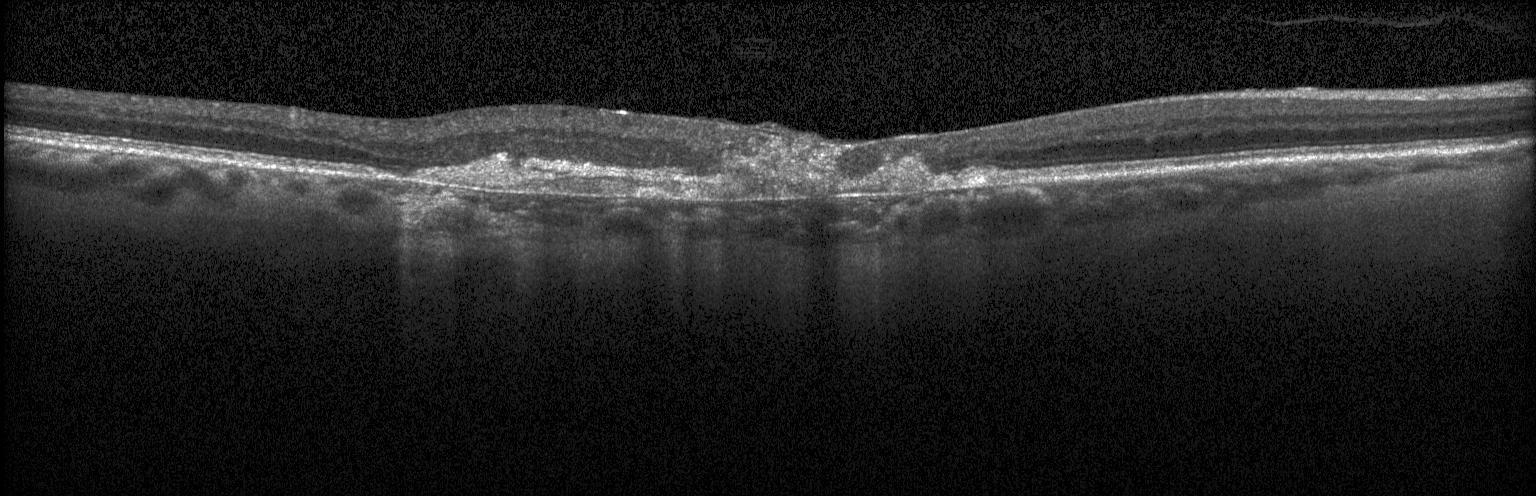

Retinal OCT B-scan; Heidelberg Spectralis OCT system; through the macula. The scan shows a choroidal neovascular membrane.